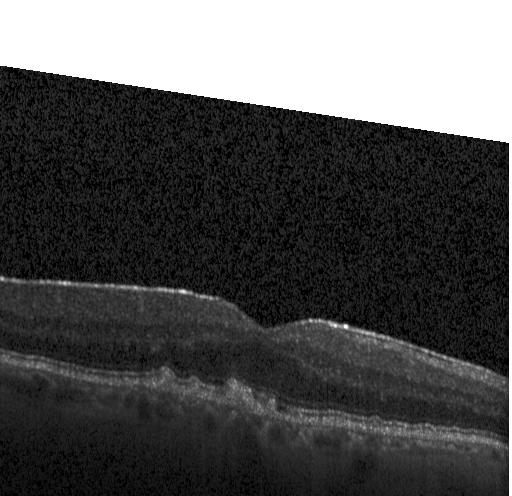
The scan shows drusen.